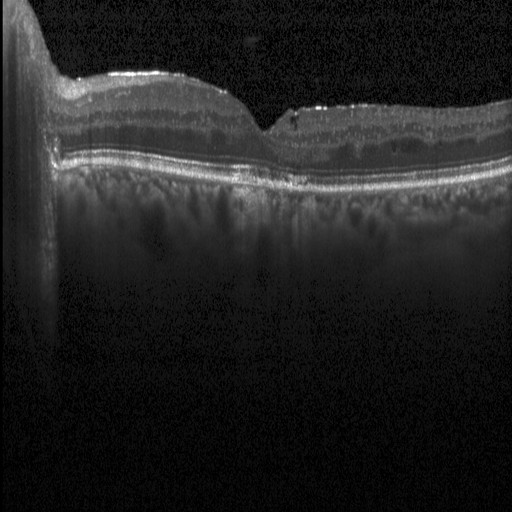
Diagnosis: diabetic macular edema (DME).